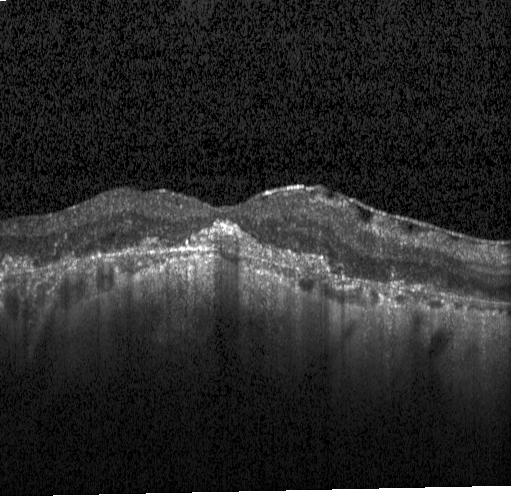
Macular OCT demonstrating choroidal neovascularization (CNV).